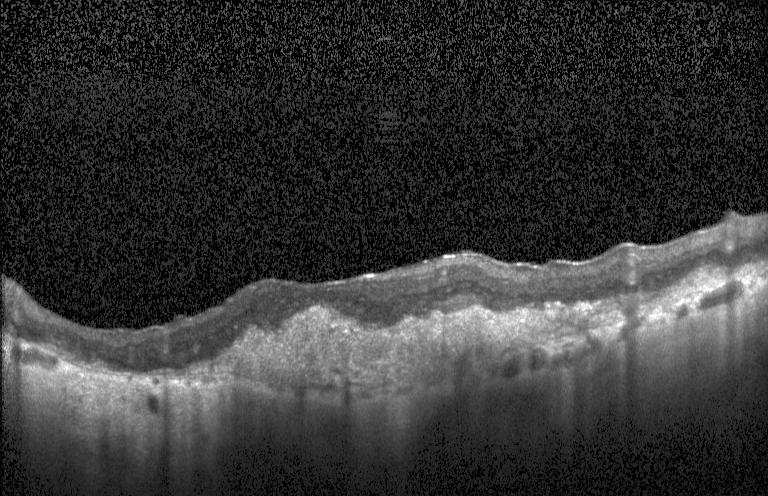 Retinal OCT cross-section · acquired on a Heidelberg Spectralis · fovea-centered. The scan shows a choroidal neovascular membrane.